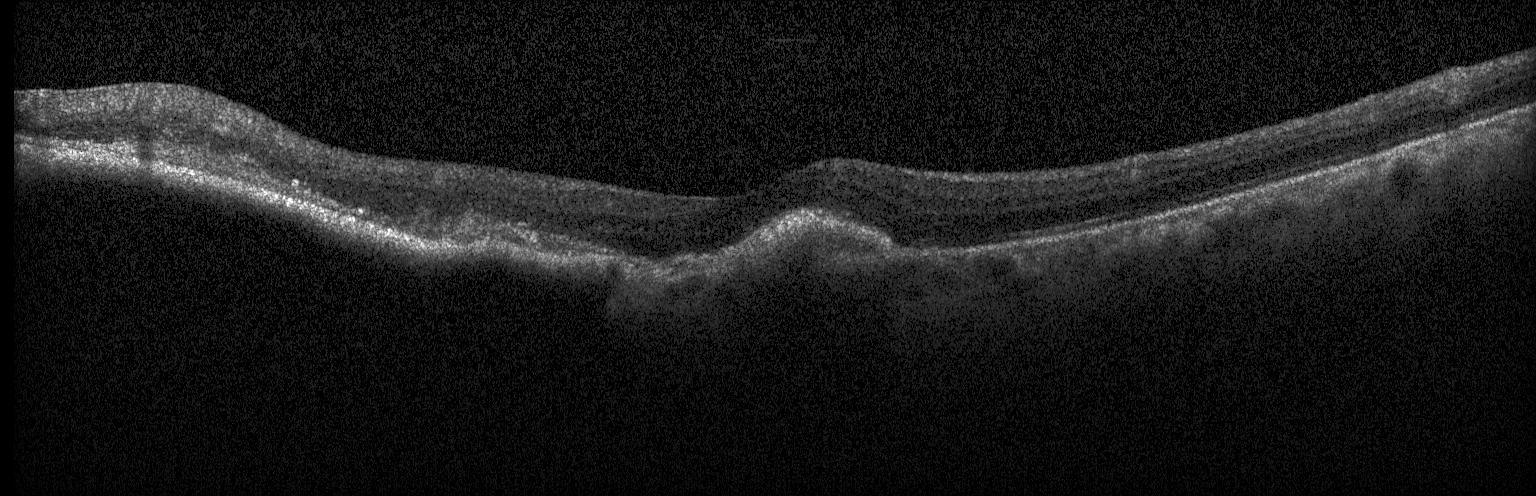
Heidelberg Spectralis, retinal OCT B-scan, fovea-centered, spectral-domain OCT — Impression: a choroidal neovascular membrane.